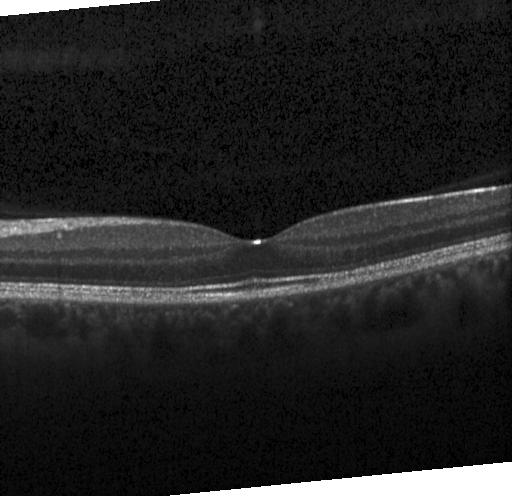
Retinal OCT B-scan. Impression: neither choroidal neovascularization, diabetic macular edema, nor drusen.